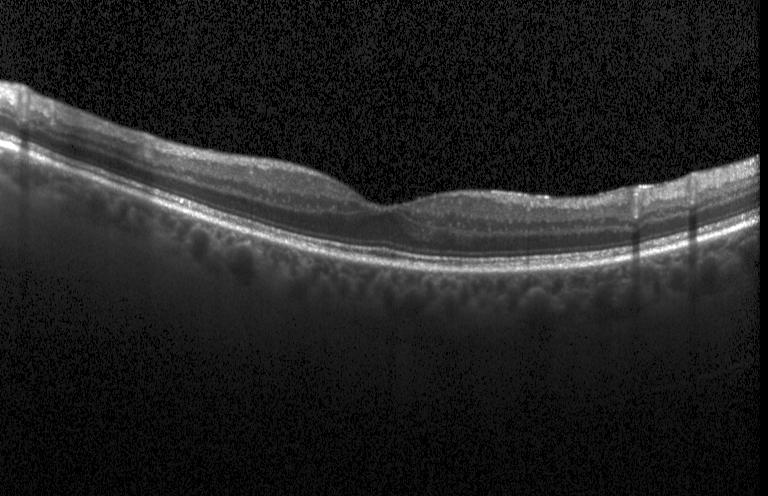

Macular scan; Heidelberg Spectralis; spectral-domain OCT; OCT B-scan
Diagnosis: neither choroidal neovascularization, diabetic macular edema, nor drusen.